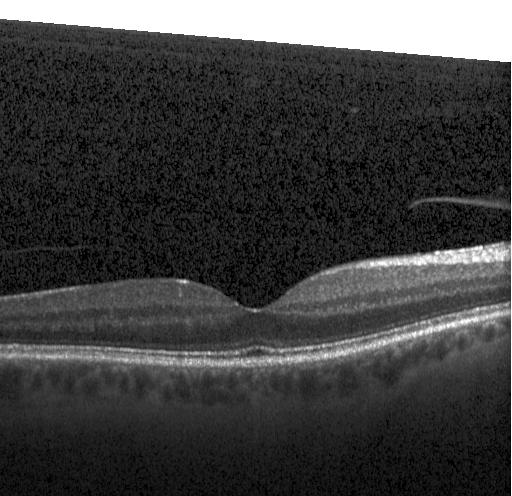 Optical coherence tomography B-scan.
Finding: no choroidal neovascularization, no diabetic macular edema, and no drusen.